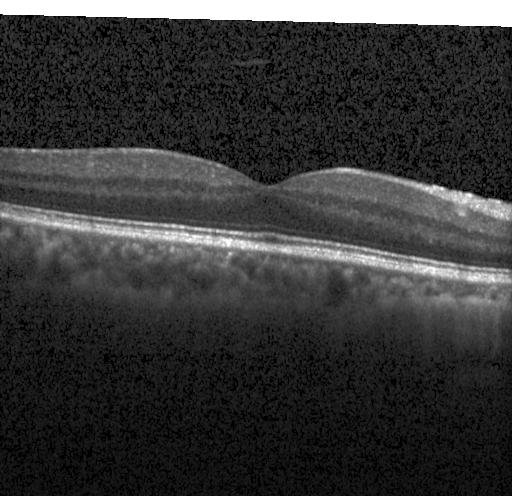
Retinal OCT B-scan
Diagnosis: no CNV, no DME, and no drusen.